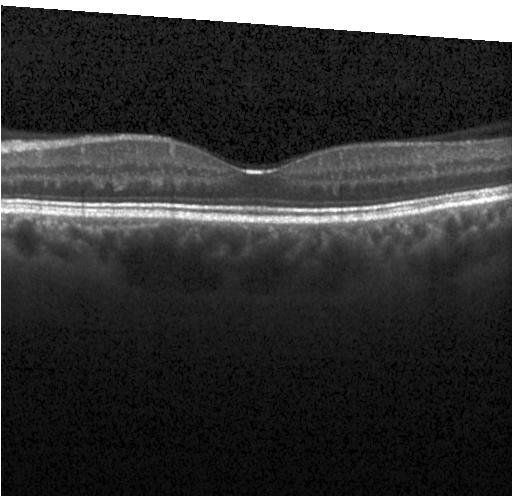 Diagnosis: no choroidal neovascularization, diabetic macular edema, or drusen.